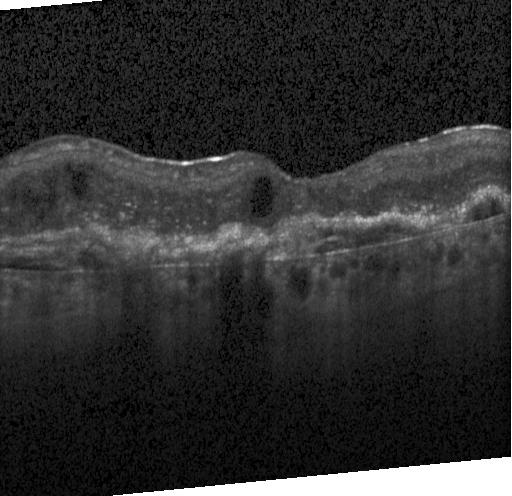
OCT B-scan. Diagnosis: a choroidal neovascular membrane.